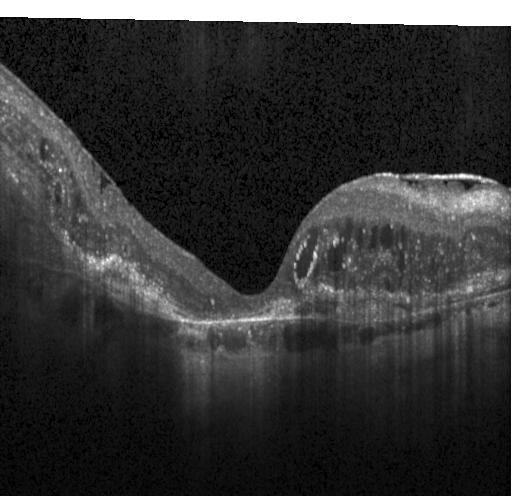

Retinal OCT cross-section · fovea-centered. The scan shows choroidal neovascularization.